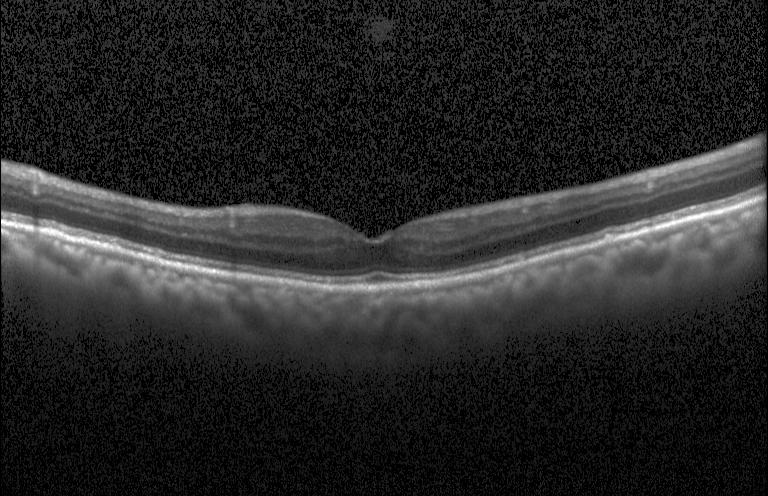 Optical coherence tomography scan — Impression: multiple drusen.